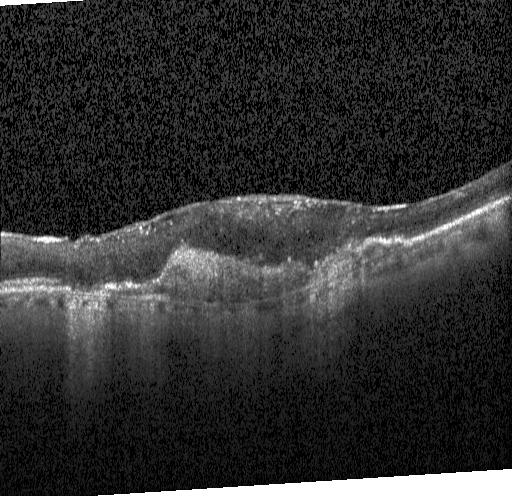
OCT scan showing CNV.